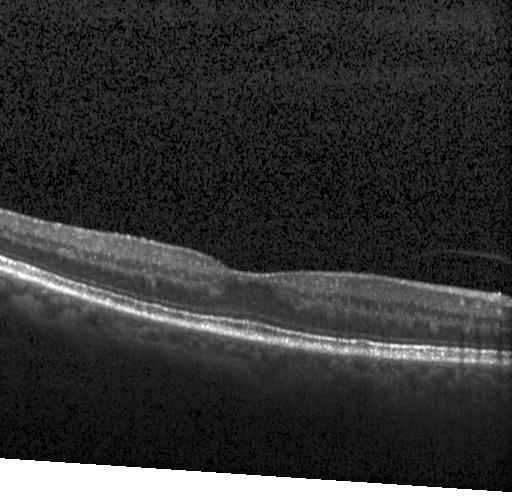

Optical coherence tomography scan — Macular OCT: no choroidal neovascularization, no diabetic macular edema, and no drusen.